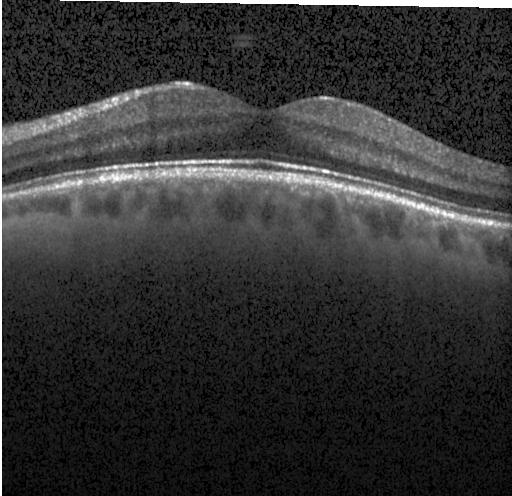

Macular OCT: neither choroidal neovascularization, diabetic macular edema, nor drusen.